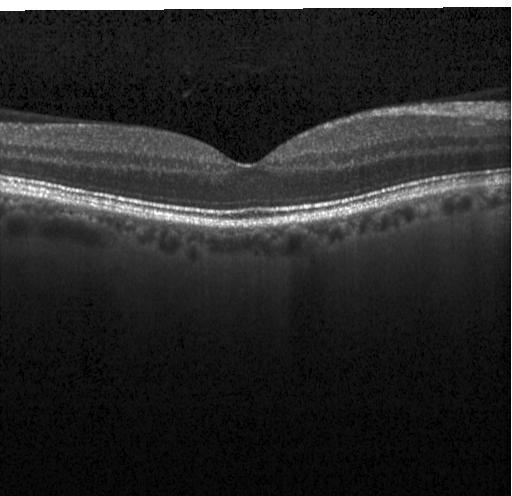

OCT line scan. Finding: no choroidal neovascularization, diabetic macular edema, or drusen.